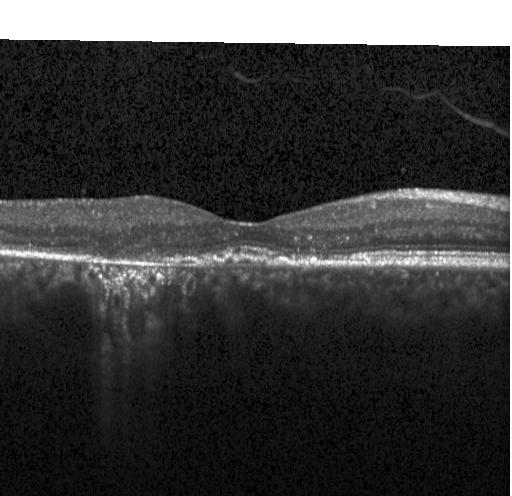 Macular OCT demonstrating choroidal neovascularization (CNV).